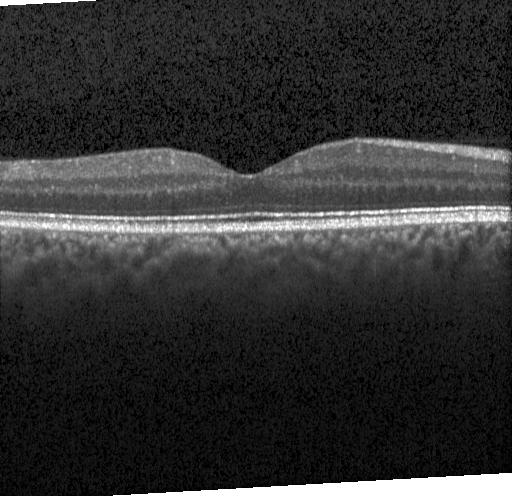

Macular scan; retinal OCT cross-section — The scan shows neither choroidal neovascularization, diabetic macular edema, nor drusen.